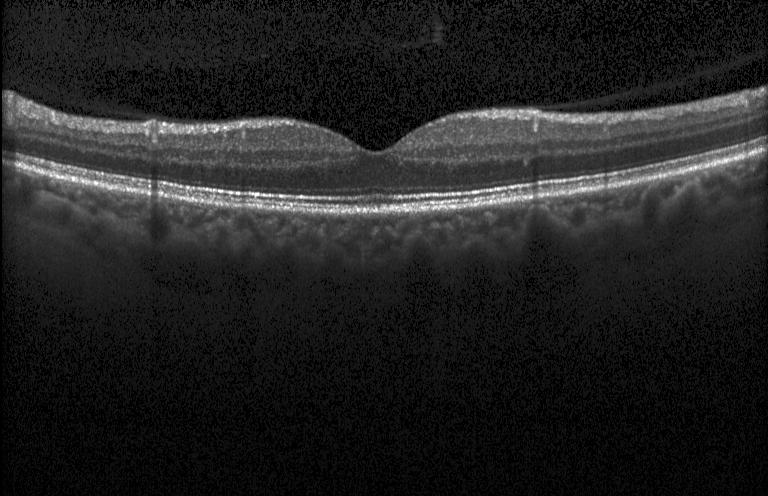
Retinal OCT cross-section, SD-OCT.
Macular OCT: neither choroidal neovascularization, diabetic macular edema, nor drusen.